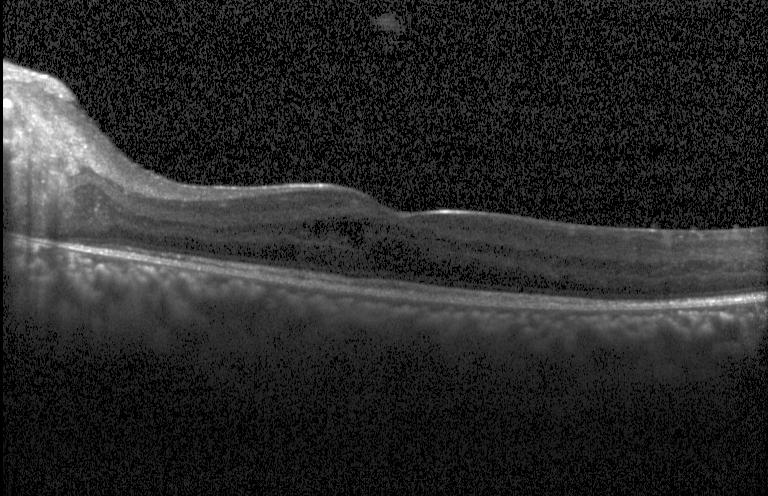
Optical coherence tomography scan
Diabetic macular edema.